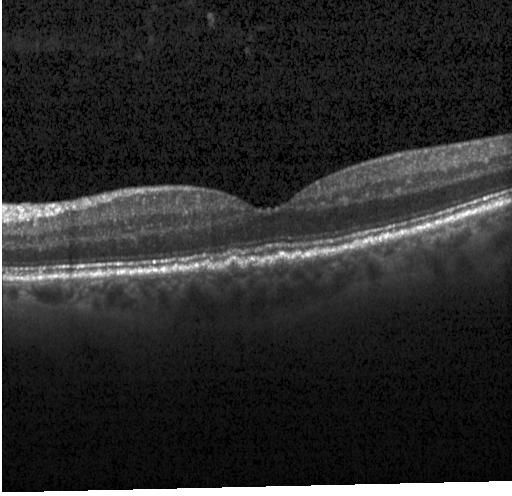
Retinal OCT B-scan — The scan shows multiple drusen.